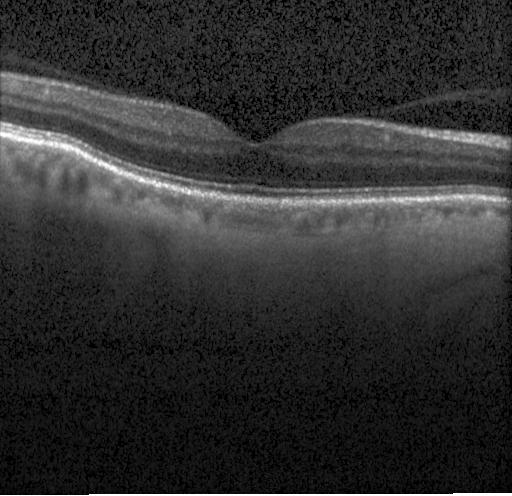

Assessment: no choroidal neovascularization, diabetic macular edema, or drusen.